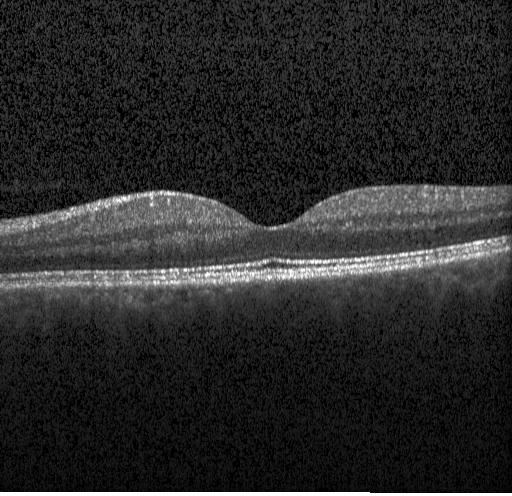
OCT B-scan · SD-OCT.
The scan shows no choroidal neovascularization, no diabetic macular edema, and no drusen.